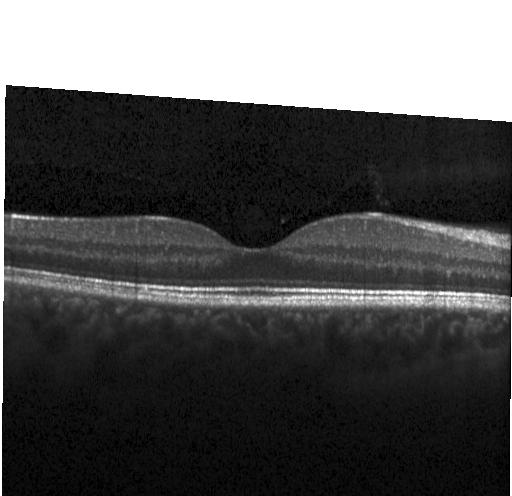
Optical coherence tomography scan. Impression: no choroidal neovascularization, diabetic macular edema, or drusen.